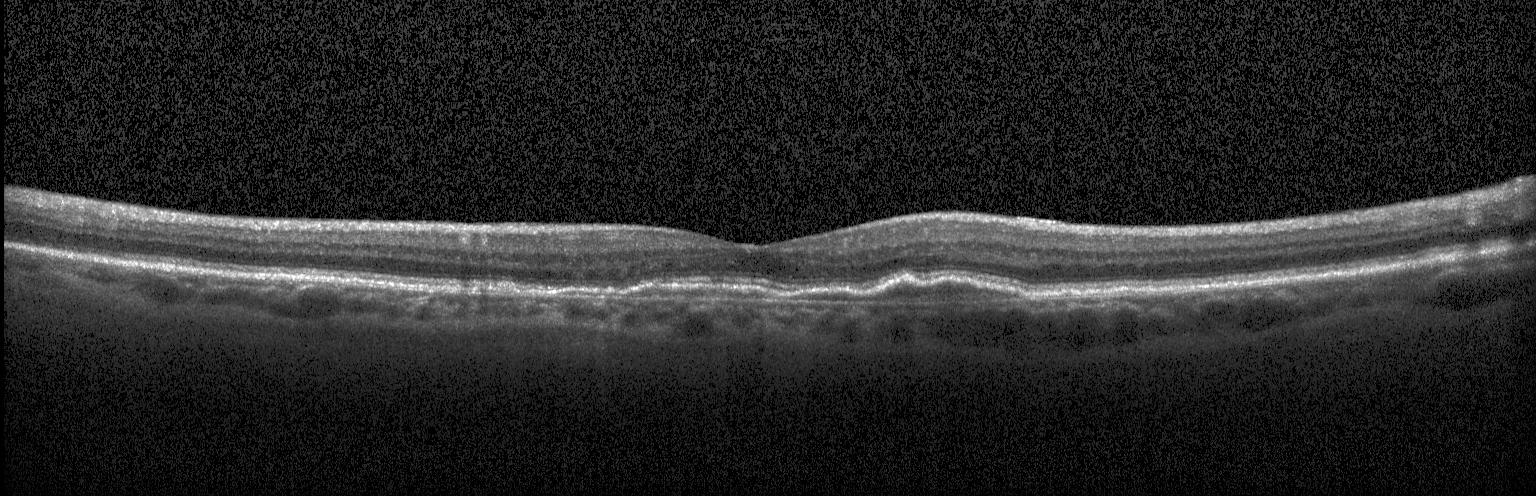
Heidelberg Spectralis · OCT line scan · spectral-domain OCT. Finding: CNV.